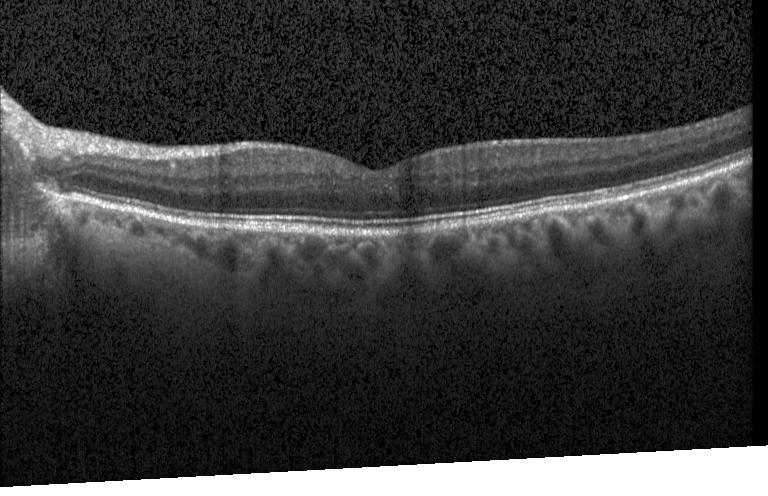

Heidelberg Spectralis; retinal OCT B-scan
Assessment: neither choroidal neovascularization, diabetic macular edema, nor drusen.